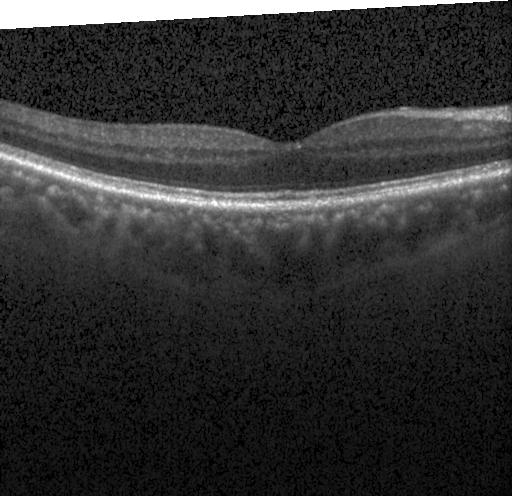 Assessment: no CNV, no DME, and no drusen.